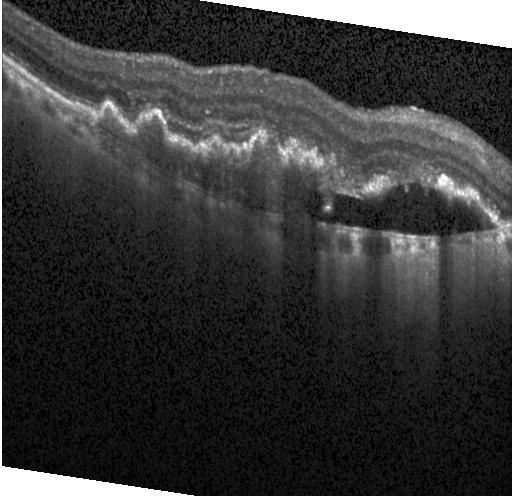

Impression: choroidal neovascularization.